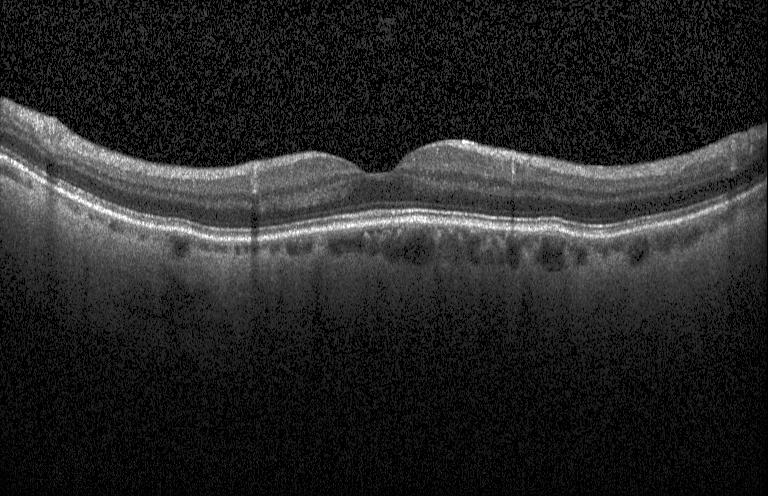
Macular OCT demonstrating neither choroidal neovascularization, diabetic macular edema, nor drusen.